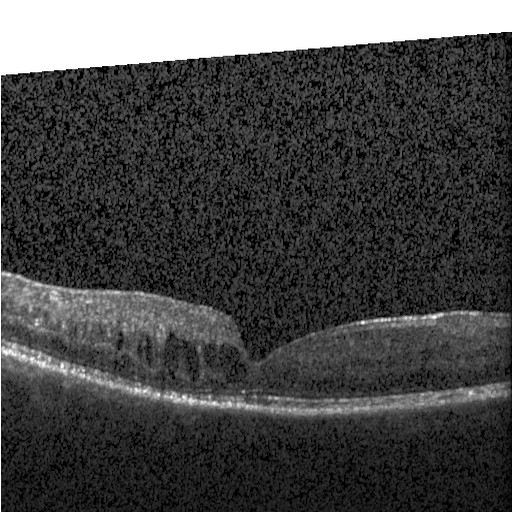

OCT line scan.
Impression: DME.